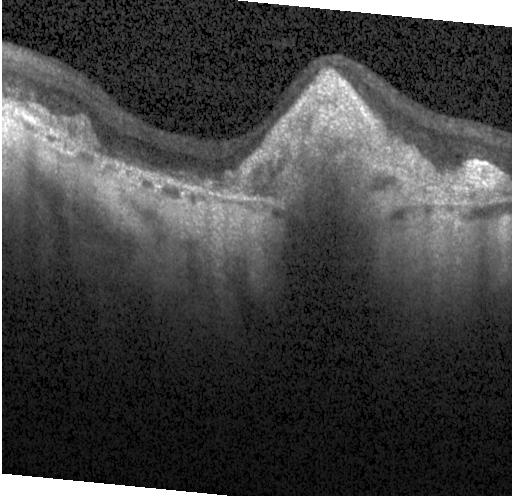

Diagnosis: CNV.